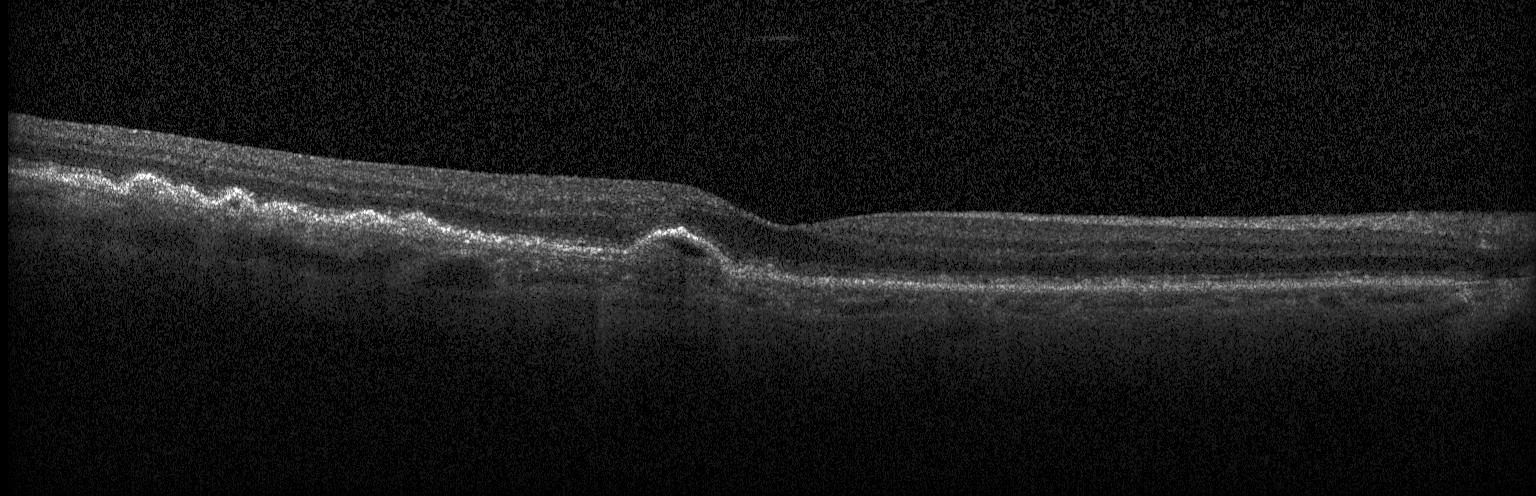 Centered on the fovea; OCT line scan. Impression: drusen.